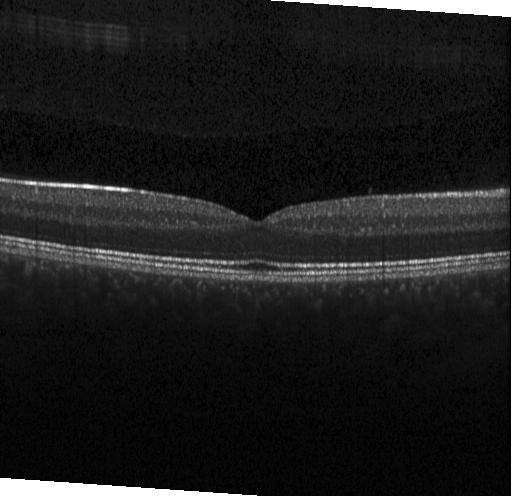
Dx: neither choroidal neovascularization, diabetic macular edema, nor drusen.